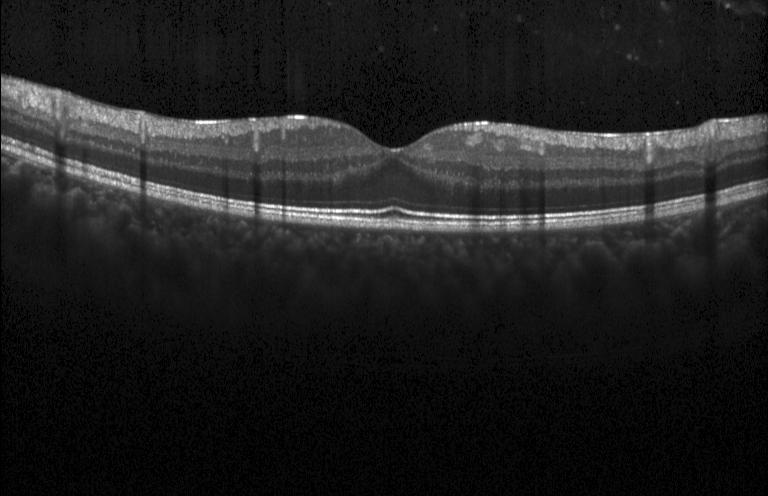 Heidelberg Spectralis · horizontal scan through the fovea · retinal OCT B-scan · spectral-domain optical coherence tomography. Assessment: no evidence of choroidal neovascularization, diabetic macular edema, or drusen.